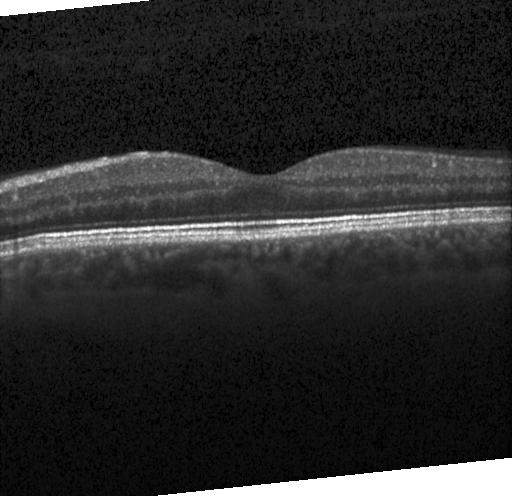

Optical coherence tomography B-scan.
This B-scan demonstrates no evidence of choroidal neovascularization, diabetic macular edema, or drusen.